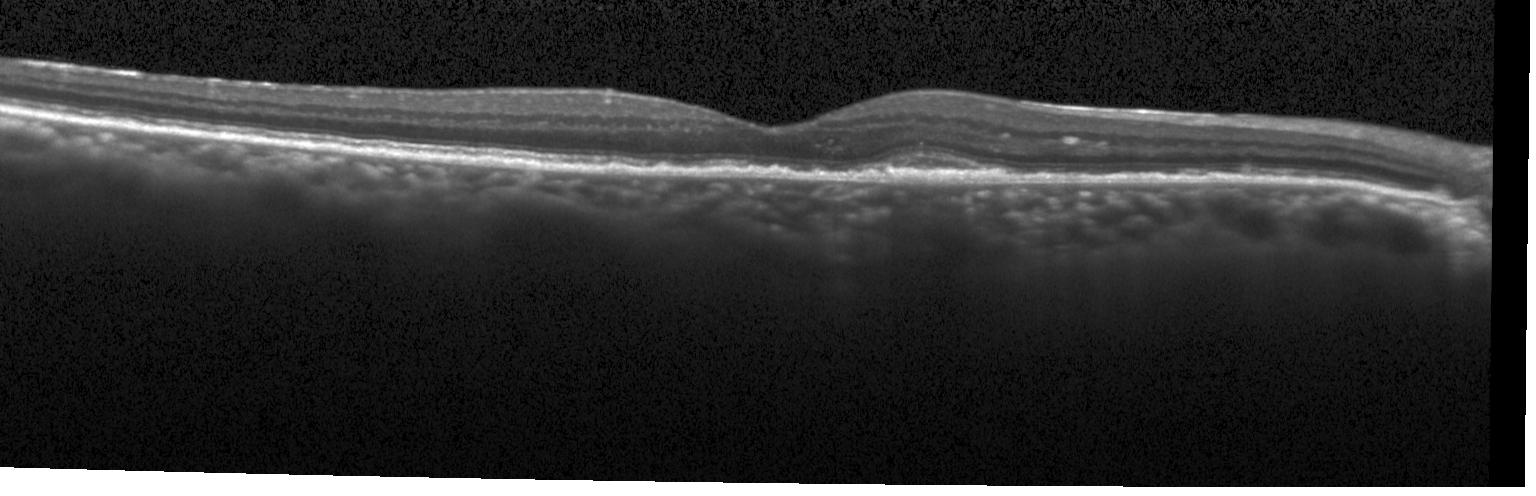

Optical coherence tomography scan; fovea-centered; acquired on a Heidelberg Spectralis
Finding: choroidal neovascularization.